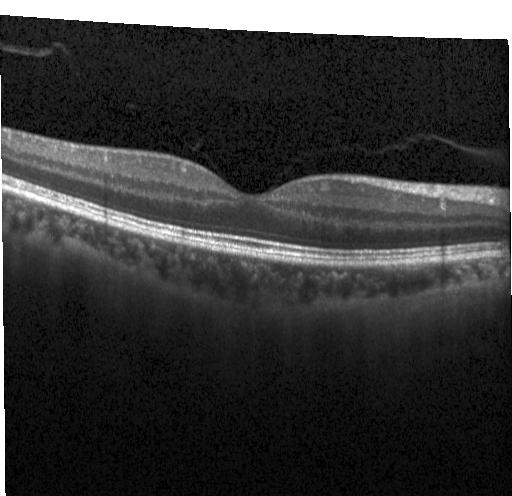 Instrument: Heidelberg Spectralis · spectral-domain OCT · horizontal scan through the fovea · retinal OCT B-scan. Dx: no CNV, no DME, and no drusen.